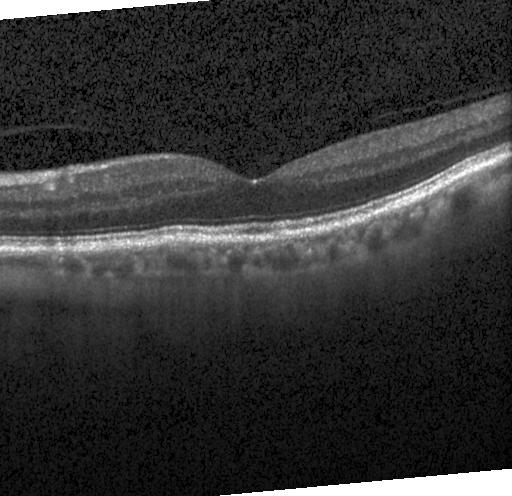

OCT scan showing no evidence of choroidal neovascularization, diabetic macular edema, or drusen.